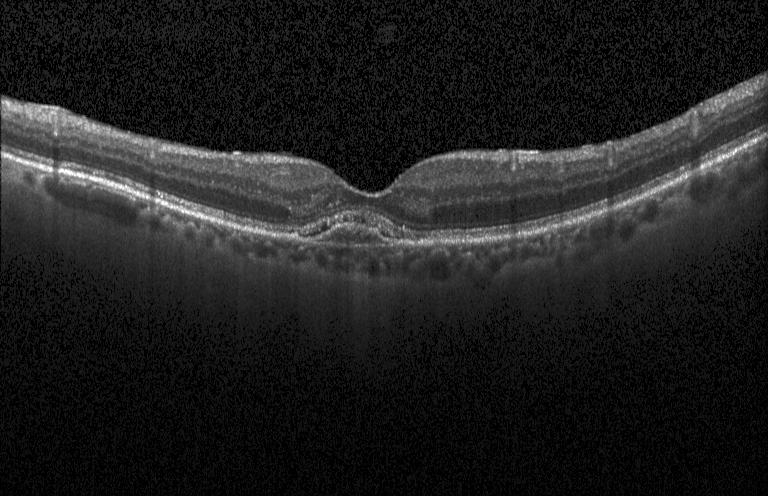 Impression: choroidal neovascularization (CNV).